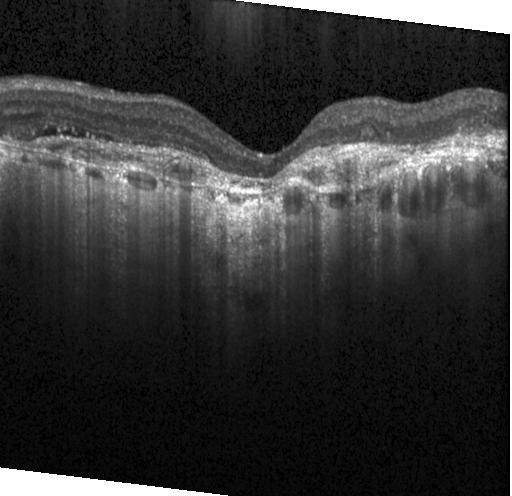 OCT B-scan showing a choroidal neovascular membrane.